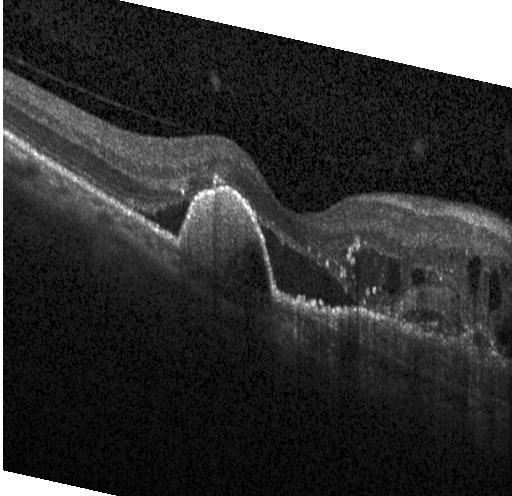
Heidelberg Spectralis; OCT B-scan; macular scan; spectral-domain OCT.
Macular OCT: a choroidal neovascular membrane.